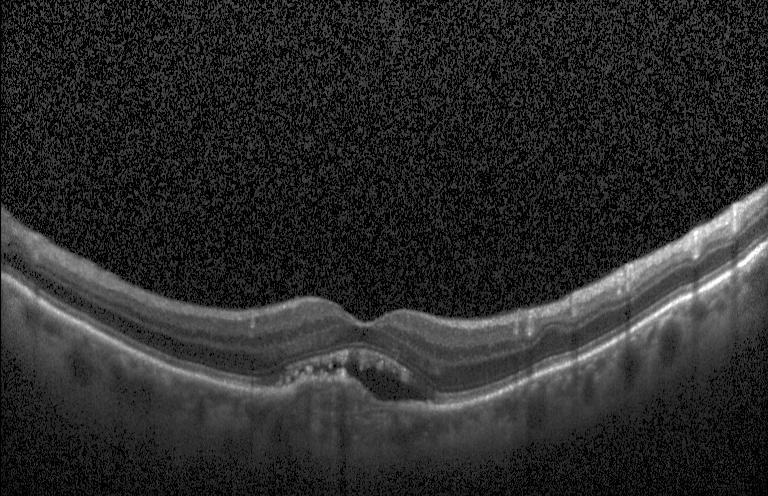

The scan shows CNV.